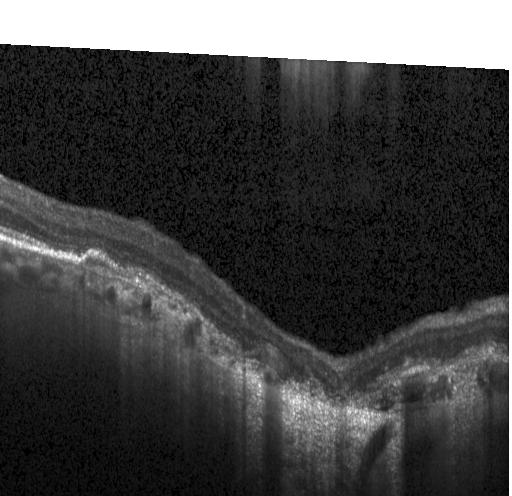 Acquired on a Heidelberg Spectralis · OCT B-scan
Assessment: a choroidal neovascular membrane.